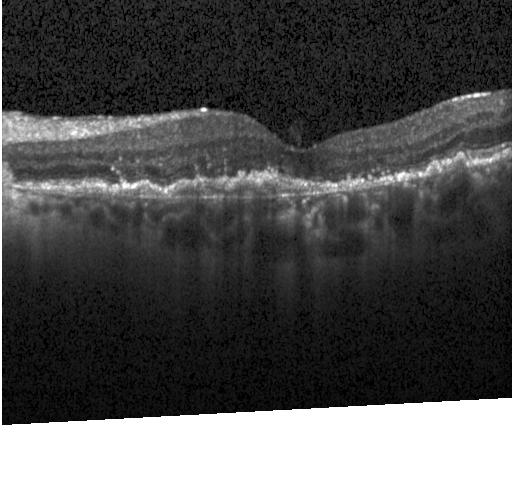 OCT line scan — Impression: a choroidal neovascular membrane.